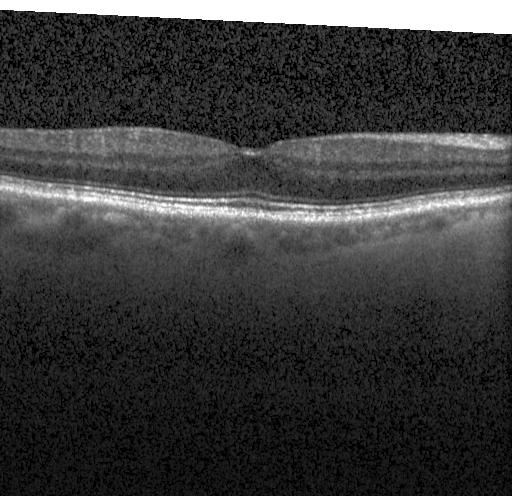

Impression: neither choroidal neovascularization, diabetic macular edema, nor drusen.